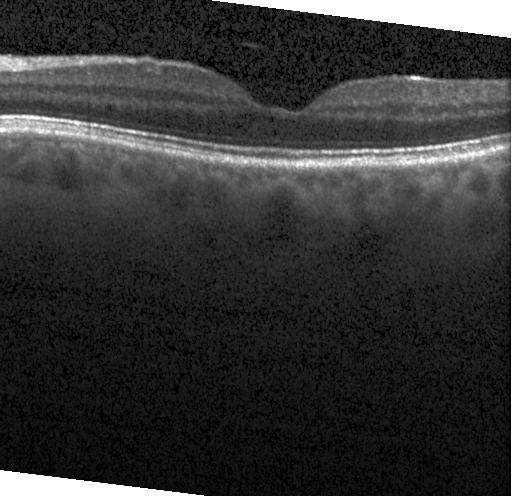
Retinal OCT B-scan — Finding: no choroidal neovascularization, no diabetic macular edema, and no drusen.